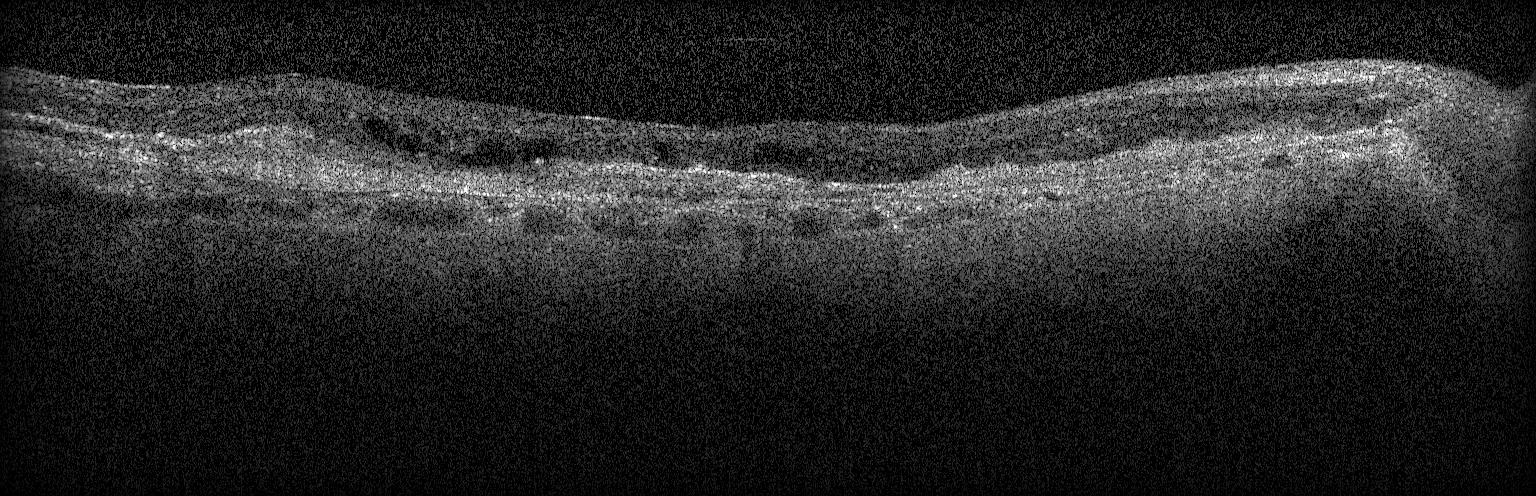

OCT finding: choroidal neovascularization (CNV).